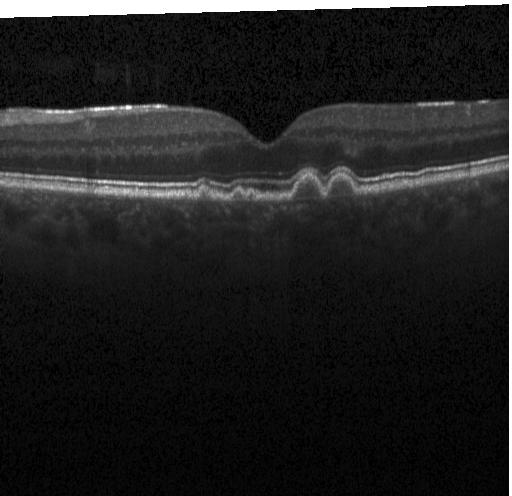

Spectral-domain optical coherence tomography · retinal OCT B-scan.
Sub-RPE drusenoid deposits.